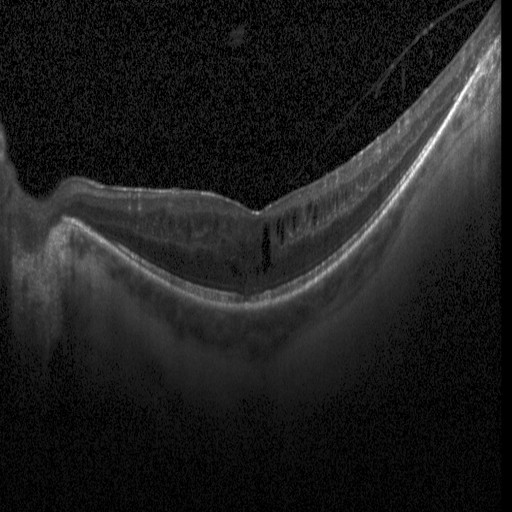 OCT line scan · horizontal scan through the fovea · spectral-domain optical coherence tomography · Heidelberg Spectralis
Diagnosis: diabetic macular edema.